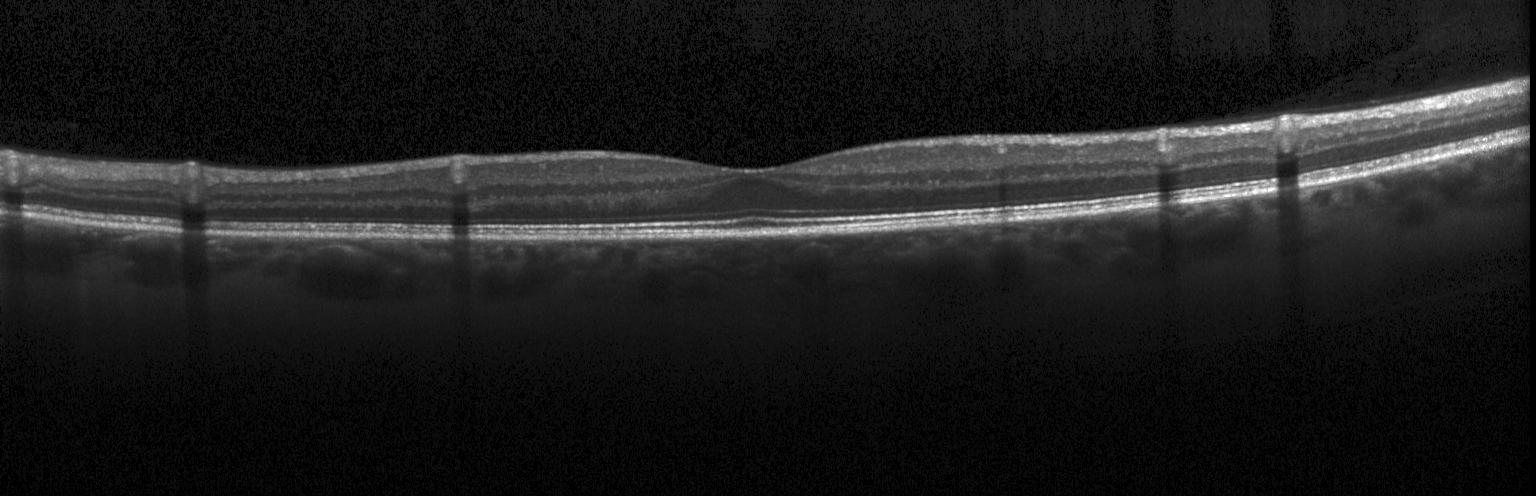

Retinal OCT B-scan; Heidelberg Spectralis; fovea-centered — Impression: neither choroidal neovascularization, diabetic macular edema, nor drusen.